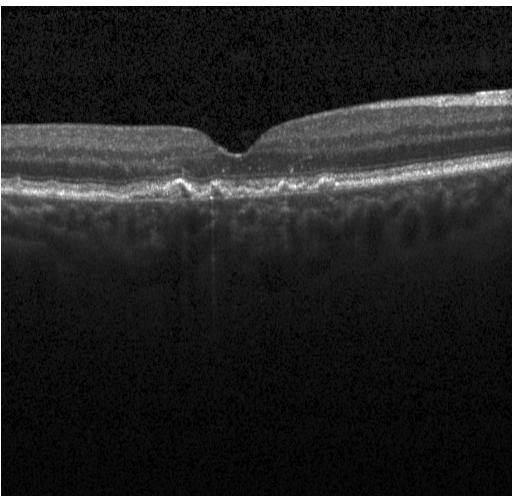
Instrument: Heidelberg Spectralis, retinal OCT cross-section. The scan shows a choroidal neovascular membrane.